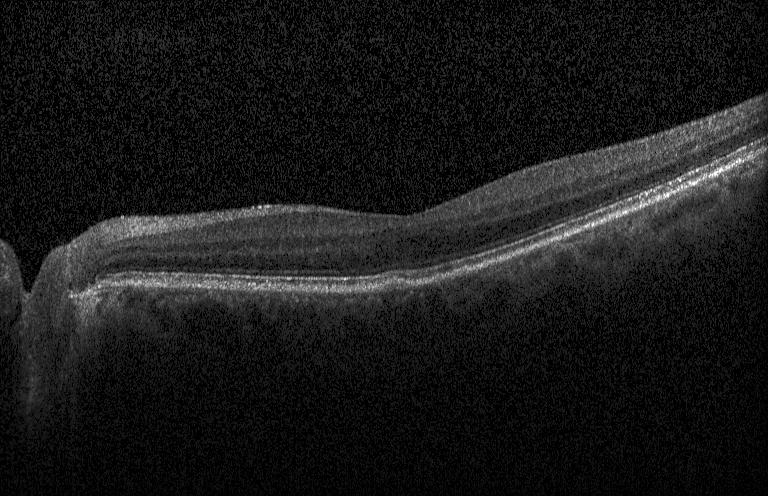

Horizontal scan through the fovea · Heidelberg Spectralis OCT system · optical coherence tomography B-scan · SD-OCT.
Impression: multiple drusen.